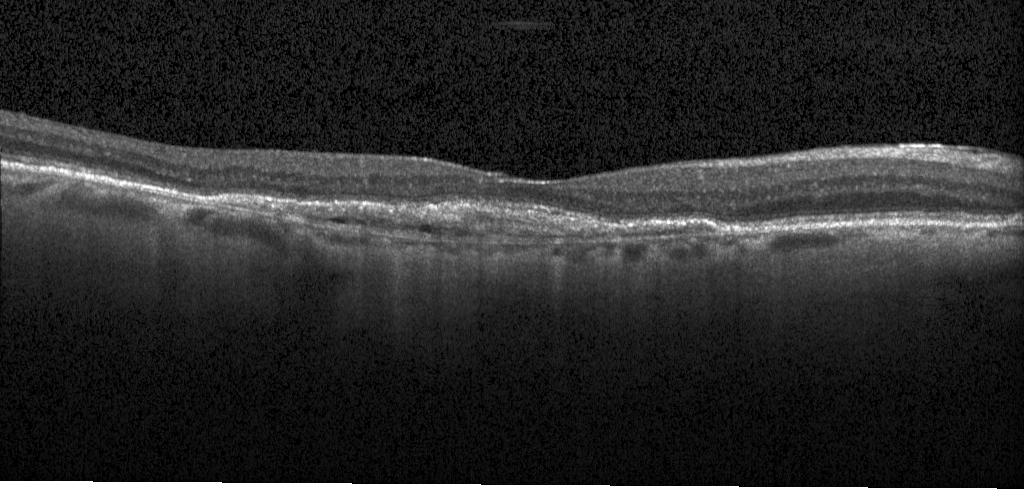 Assessment: a choroidal neovascular membrane.